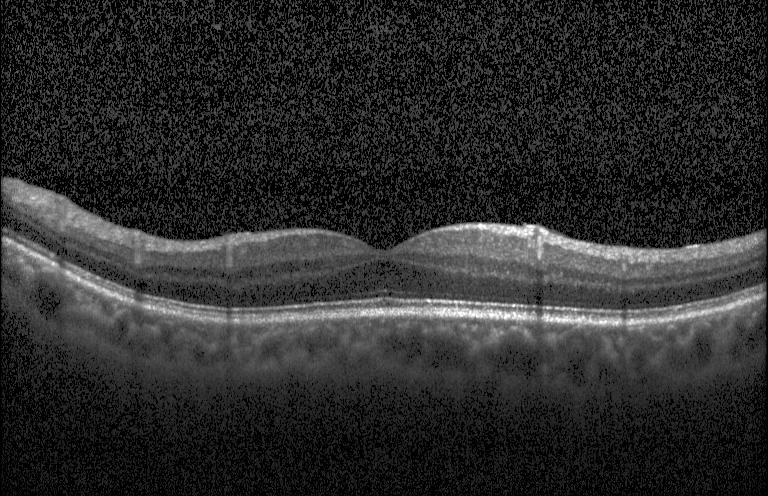 Retinal OCT cross-section. SD-OCT. Centered on the fovea. Heidelberg Spectralis
Diagnosis: no CNV, DME, or drusen.